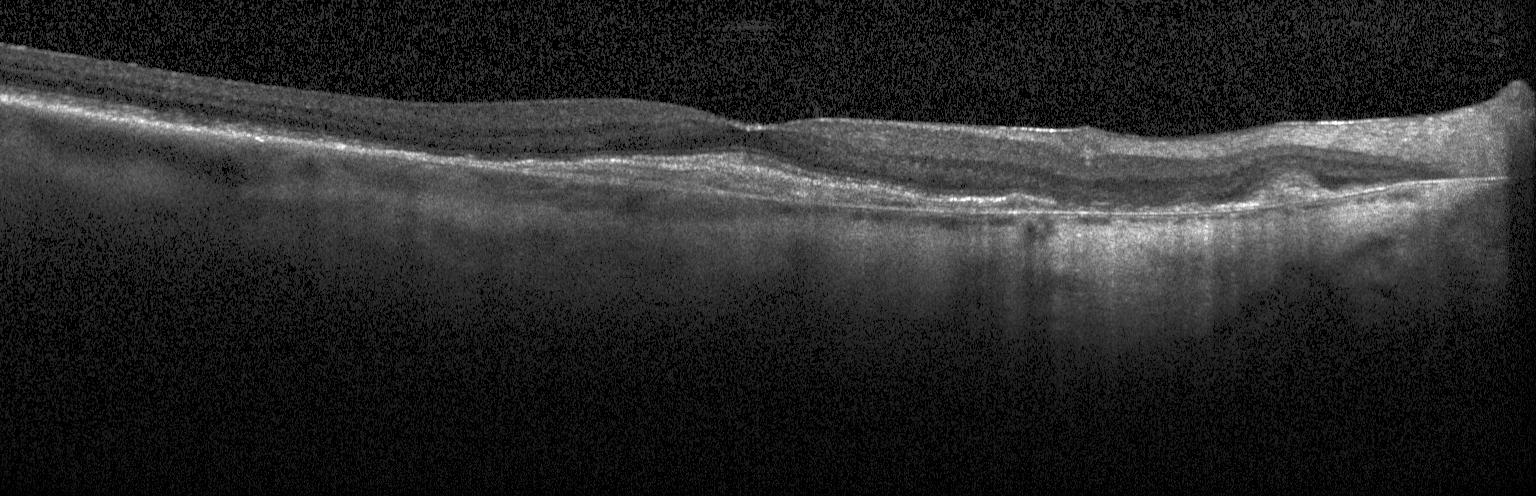 Diagnosis: a choroidal neovascular membrane.